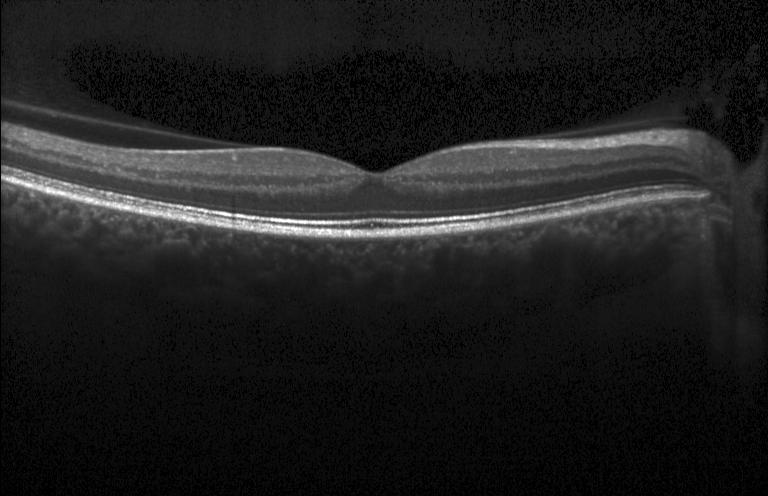
OCT finding: no choroidal neovascularization, no diabetic macular edema, and no drusen.